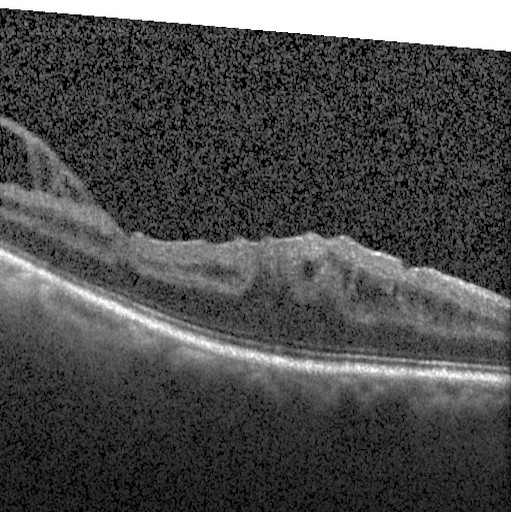 Spectral-domain optical coherence tomography. OCT B-scan. Instrument: Heidelberg Spectralis — Finding: diabetic macular edema.